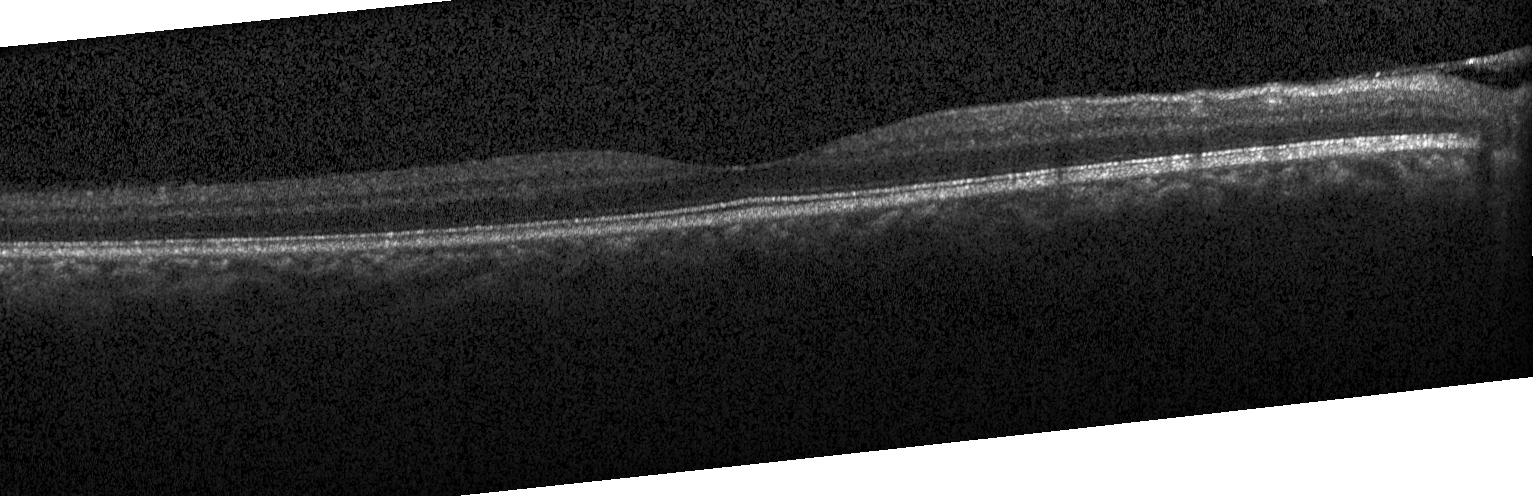

Diagnosis: no choroidal neovascularization, no diabetic macular edema, and no drusen.